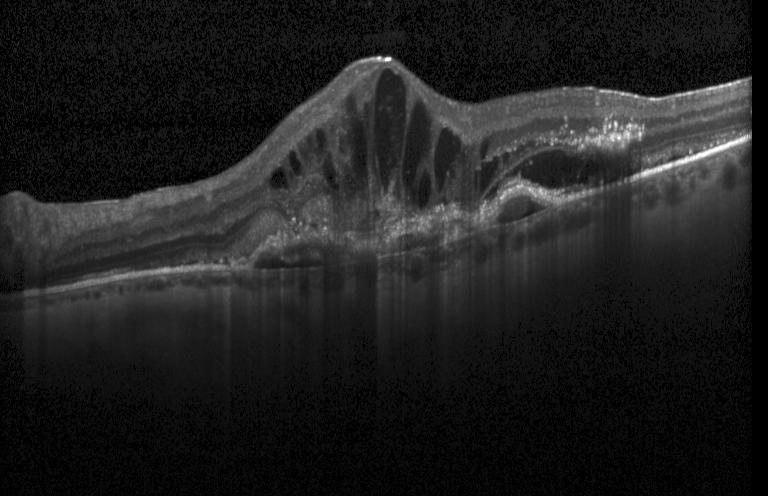
Diagnosis: CNV.